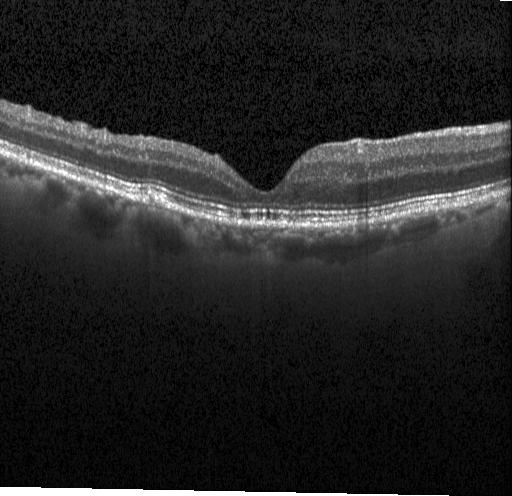

Finding: sub-RPE drusenoid deposits.